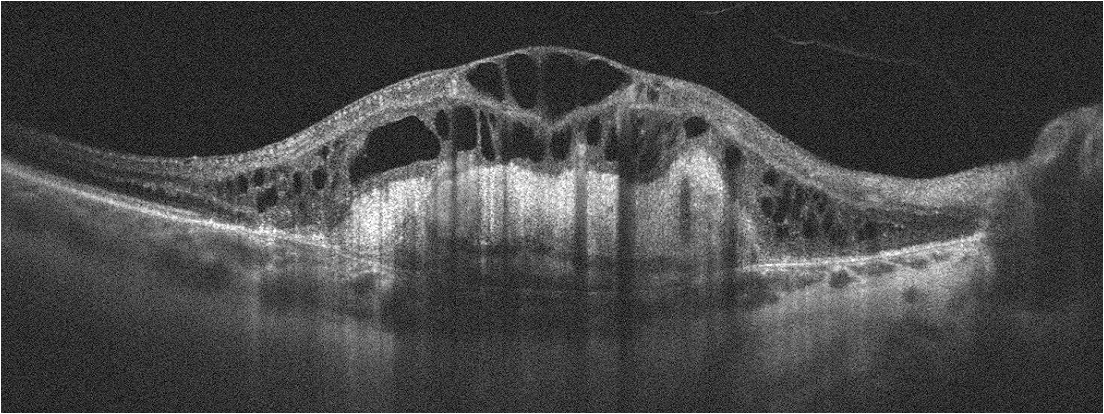

Retinal OCT cross-section. Acquired on an Optovue Avanti RTVue XR. Macular OCT: AMD.